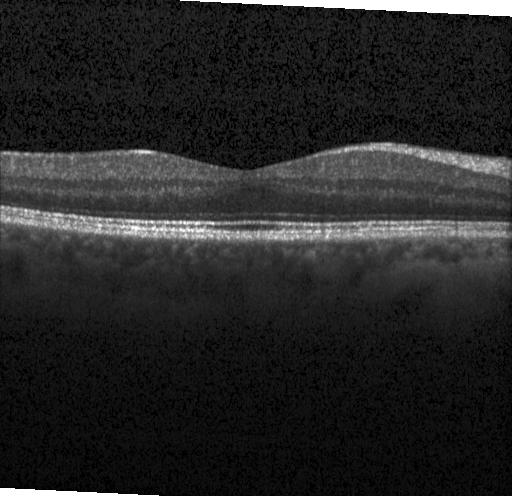
Finding: no evidence of choroidal neovascularization, diabetic macular edema, or drusen.